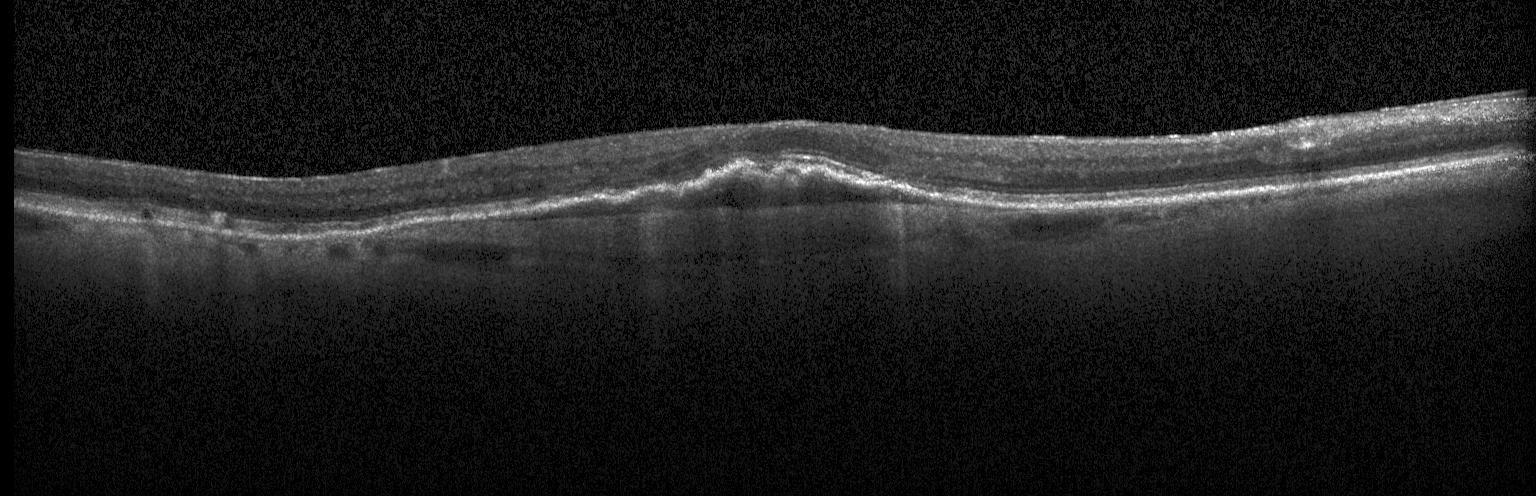 Assessment: a choroidal neovascular membrane.